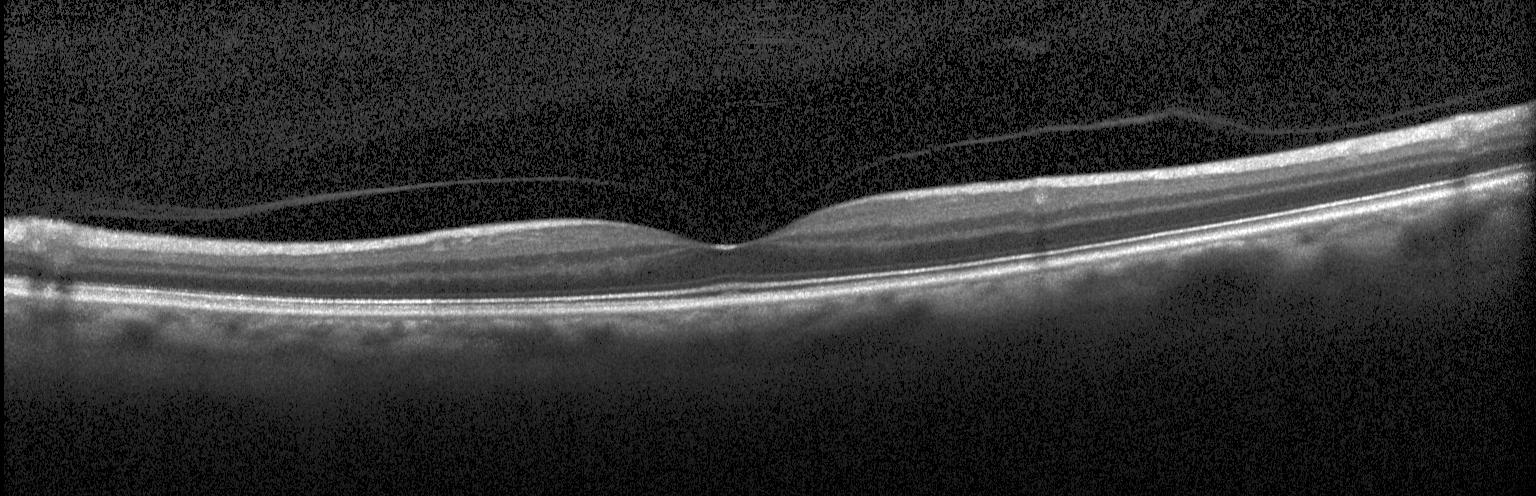 No choroidal neovascularization, diabetic macular edema, or drusen.